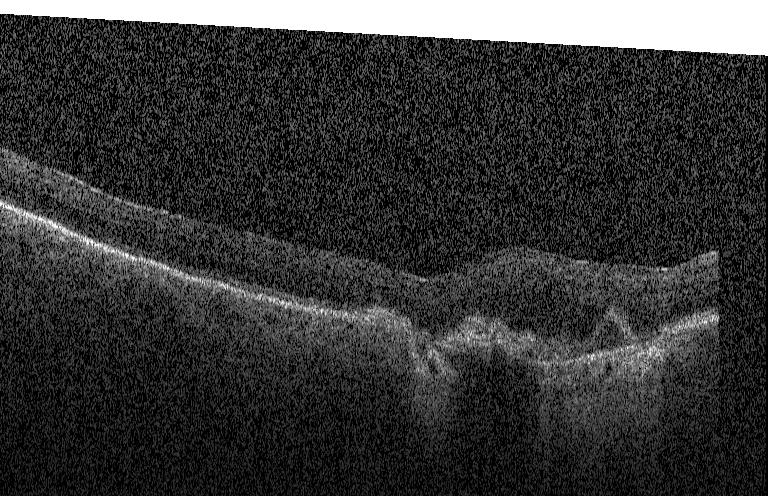

OCT B-scan showing a choroidal neovascular membrane.